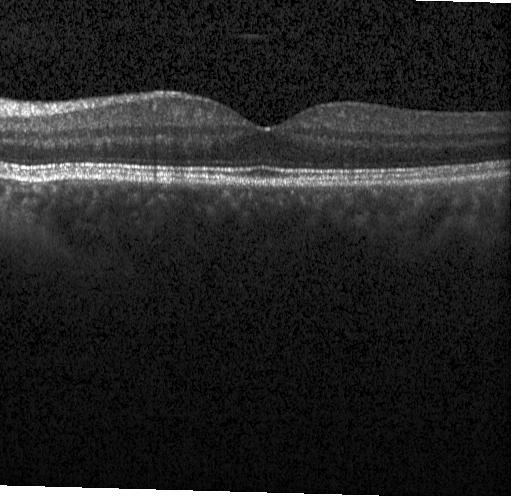
Optical coherence tomography B-scan, instrument: Heidelberg Spectralis, spectral-domain optical coherence tomography
Assessment: no choroidal neovascularization, diabetic macular edema, or drusen.